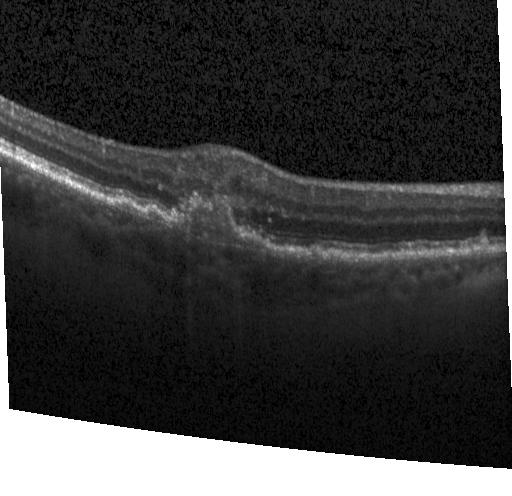
Macular OCT: choroidal neovascularization (CNV).